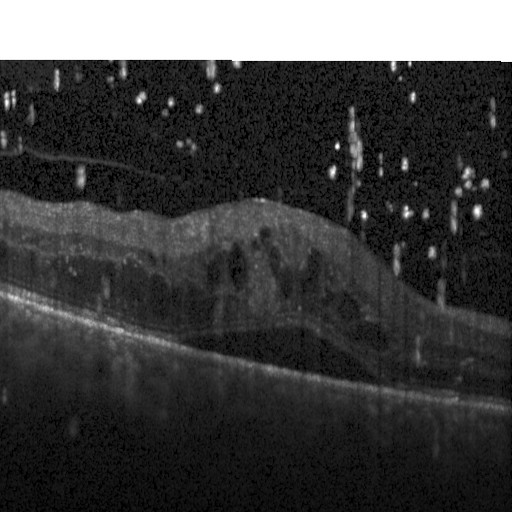

OCT finding: diabetic macular edema.